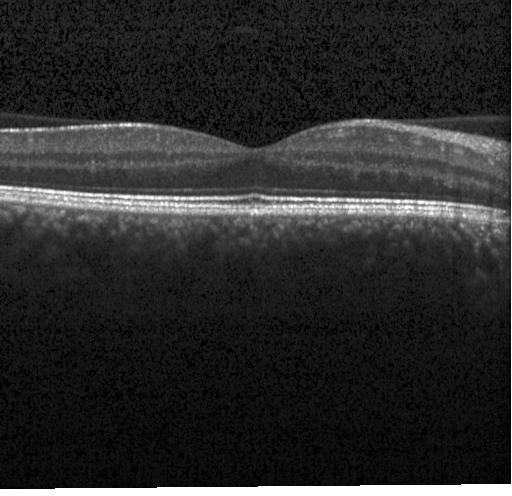

Through the macula, retinal OCT cross-section, spectral-domain OCT, acquired on a Heidelberg Spectralis
Neither CNV, DME, nor drusen.